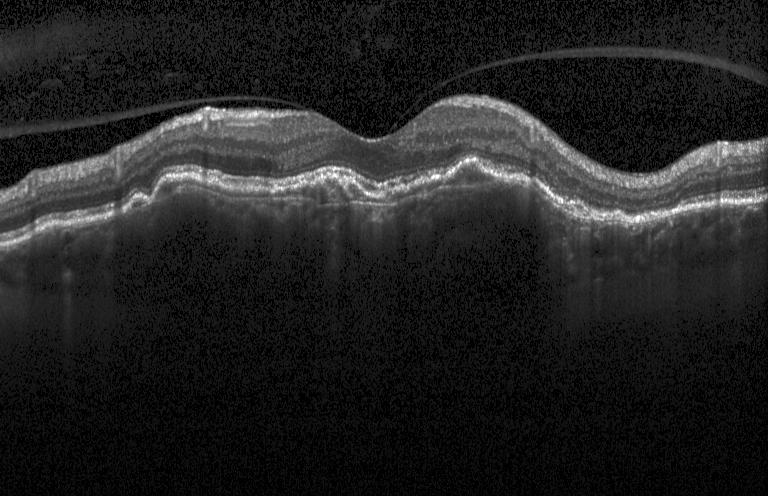

Centered on the fovea, retinal OCT B-scan, Heidelberg Spectralis OCT system, SD-OCT. This B-scan demonstrates a choroidal neovascular membrane.